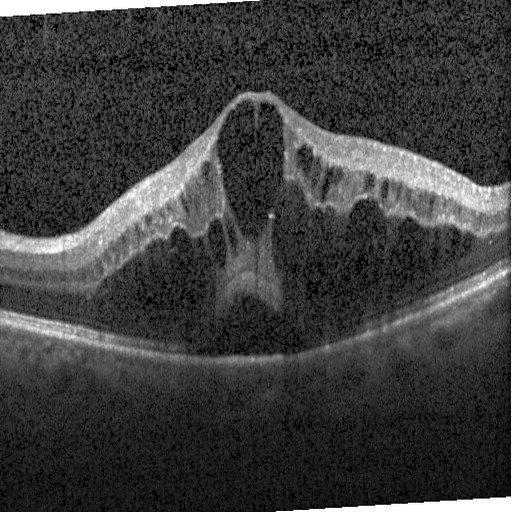 Through the macula. SD-OCT. OCT line scan. Heidelberg Spectralis. Macular OCT: DME.